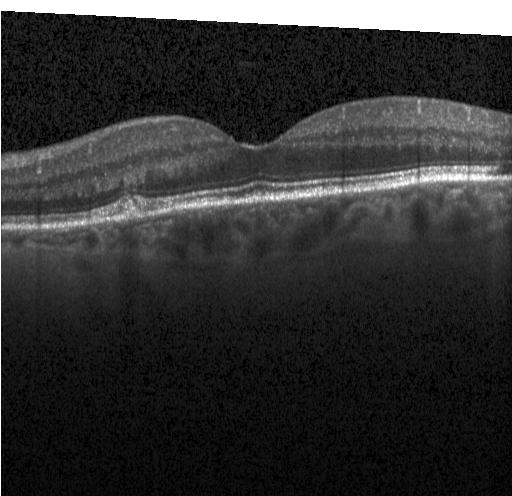
Multiple drusen.